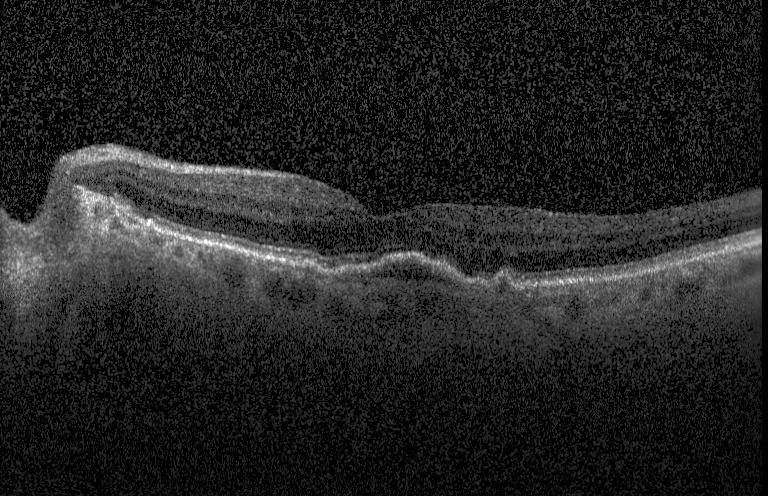
Retinal OCT B-scan. Impression: a choroidal neovascular membrane.